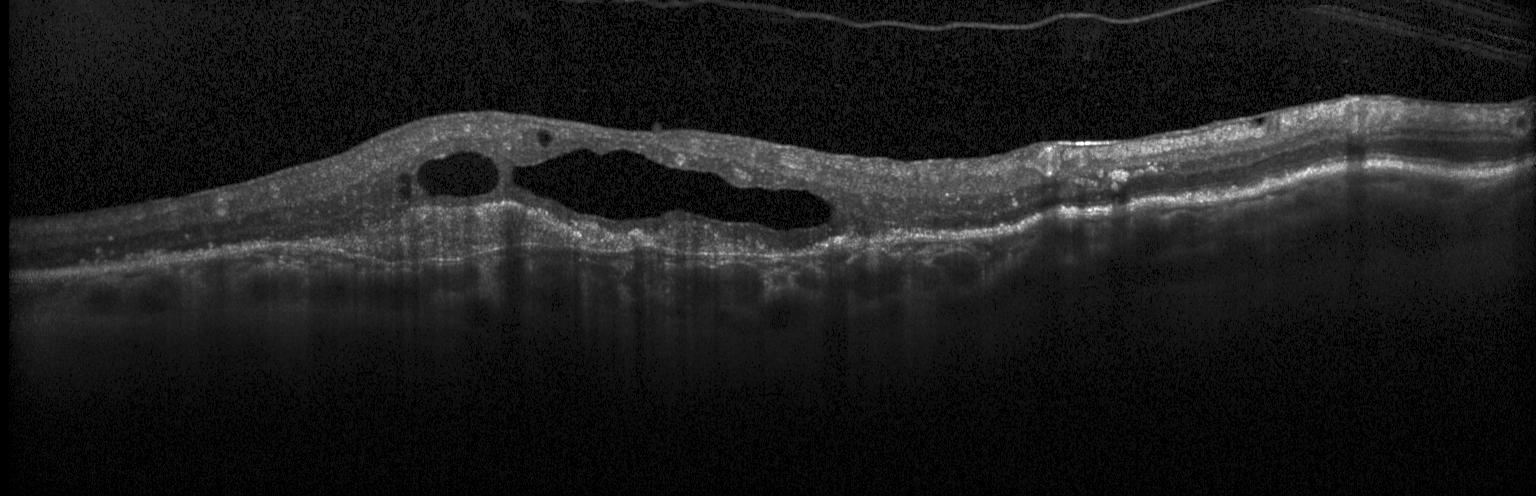

Dx: a choroidal neovascular membrane.